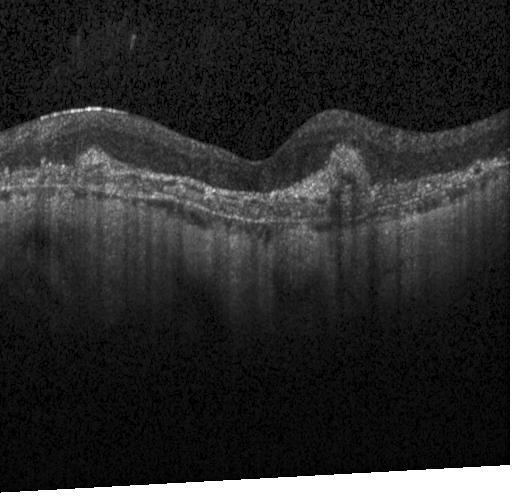
Impression: a choroidal neovascular membrane.